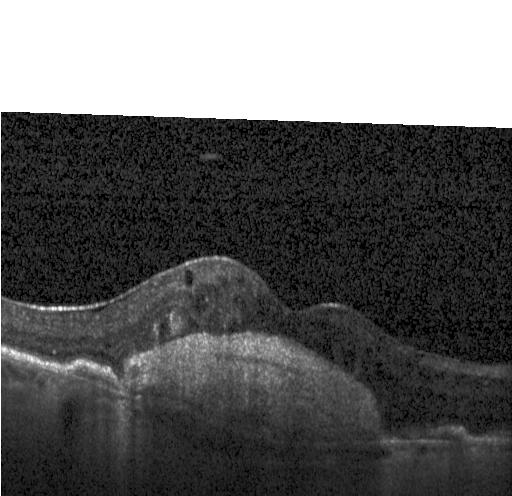 Retinal OCT cross-section, spectral-domain OCT, acquired on a Heidelberg Spectralis, horizontal scan through the fovea.
This B-scan demonstrates a choroidal neovascular membrane.